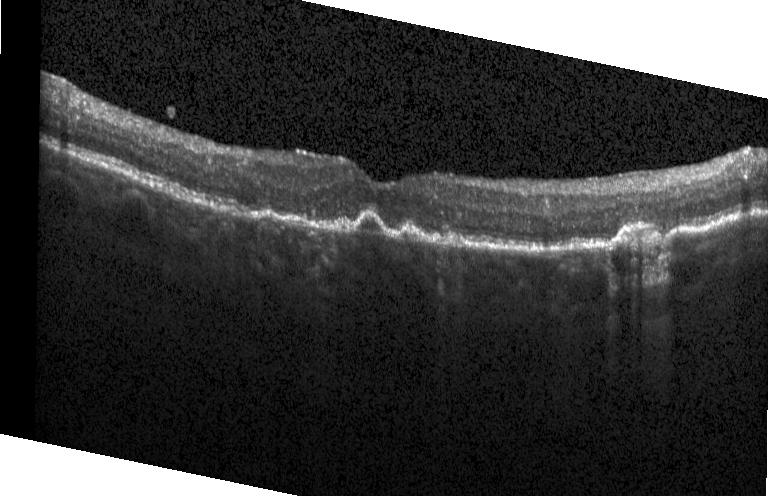
Centered on the fovea. OCT line scan. Spectral-domain optical coherence tomography.
Diagnosis: CNV.